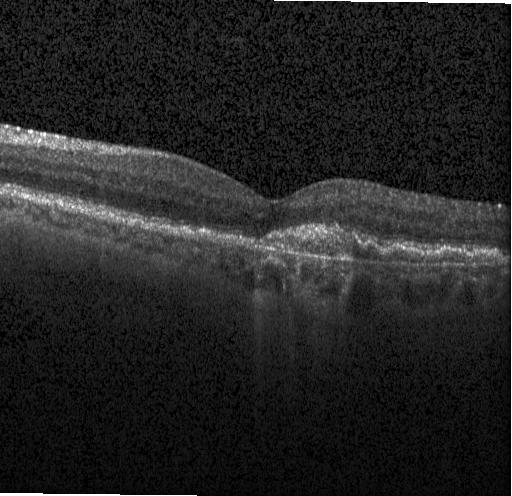 Retinal OCT cross-section showing CNV.